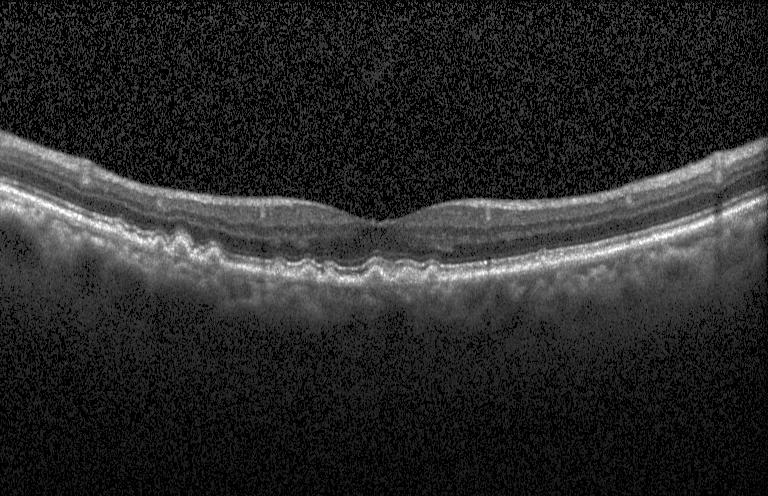

Through the macula · OCT B-scan
The scan shows drusen.